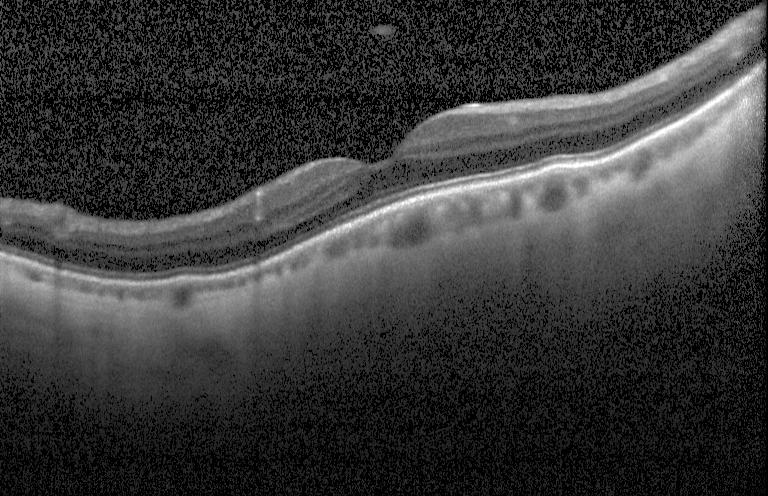 Macular OCT: no evidence of choroidal neovascularization, diabetic macular edema, or drusen.